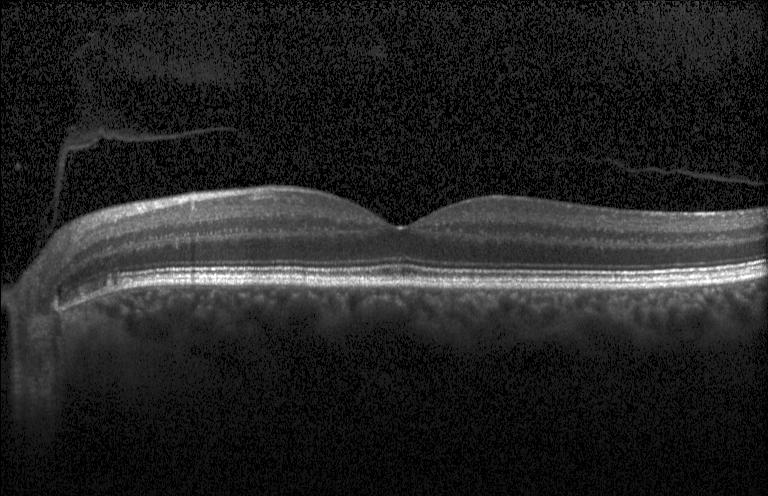

Spectral-domain OCT. OCT line scan. Macular OCT: neither CNV, DME, nor drusen.